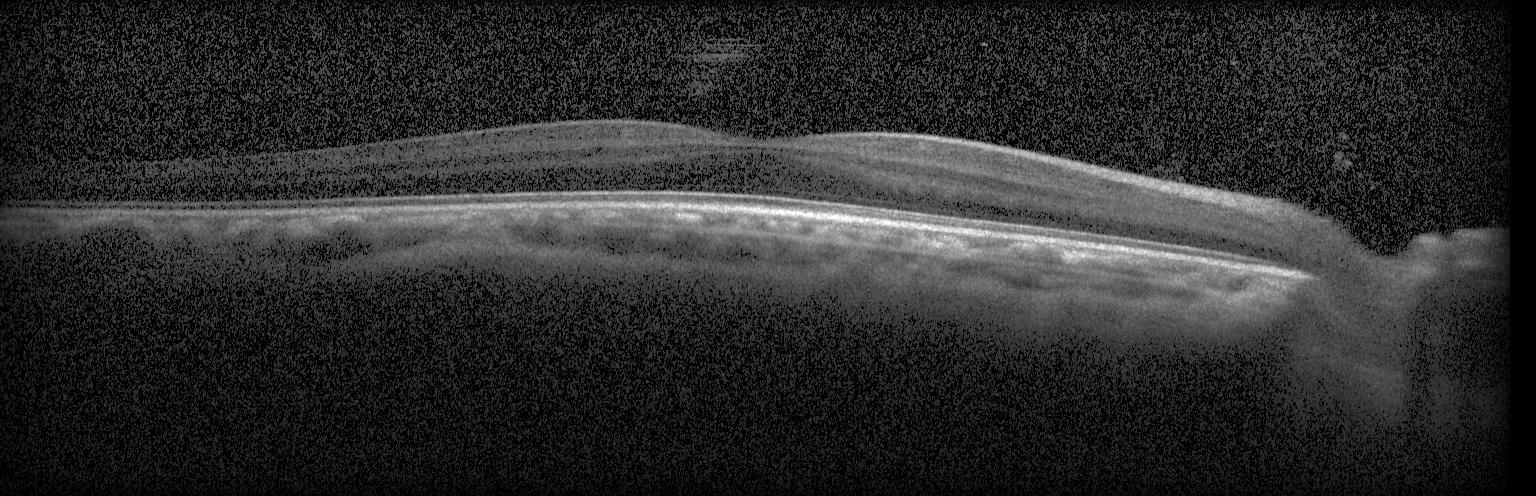
Retinal OCT cross-section.
Finding: neither CNV, DME, nor drusen.